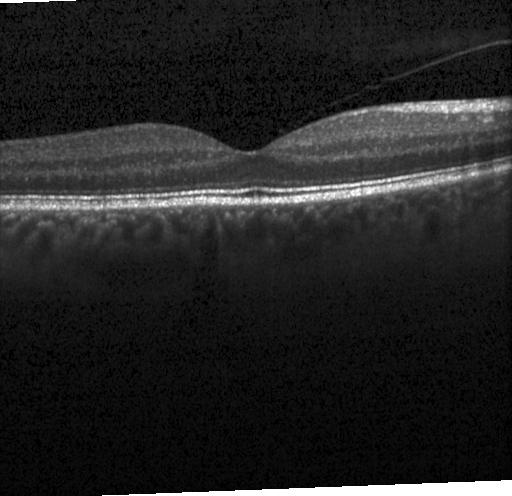 Fovea-centered; optical coherence tomography scan; Heidelberg Spectralis. Neither choroidal neovascularization, diabetic macular edema, nor drusen.